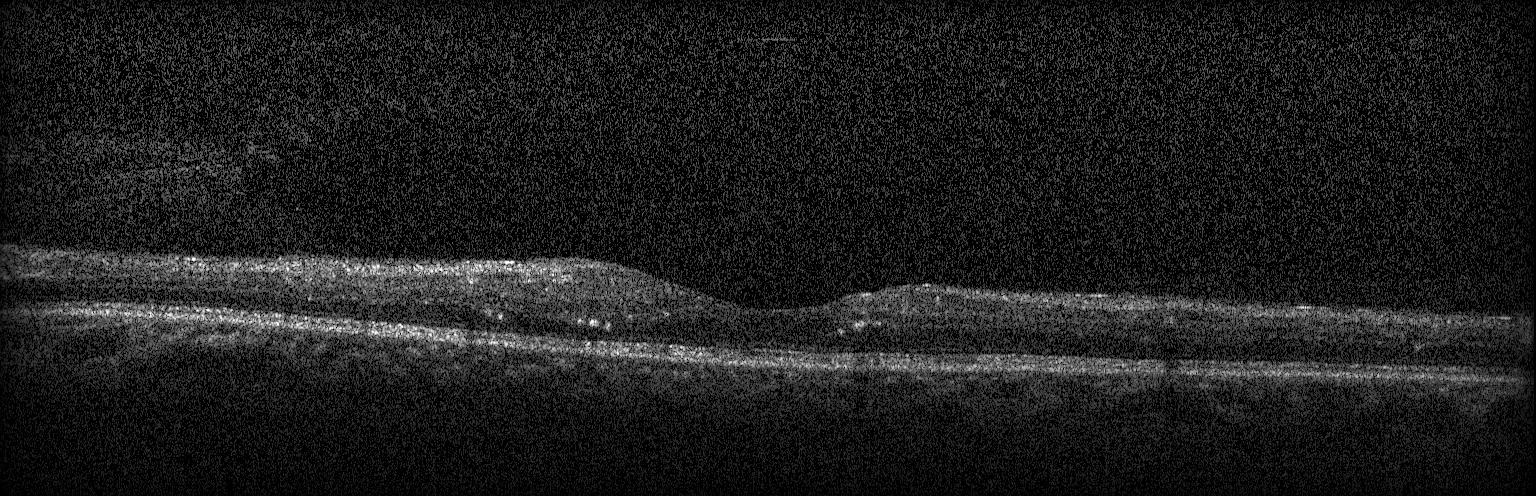
Retinal OCT B-scan.
Finding: diabetic macular edema.